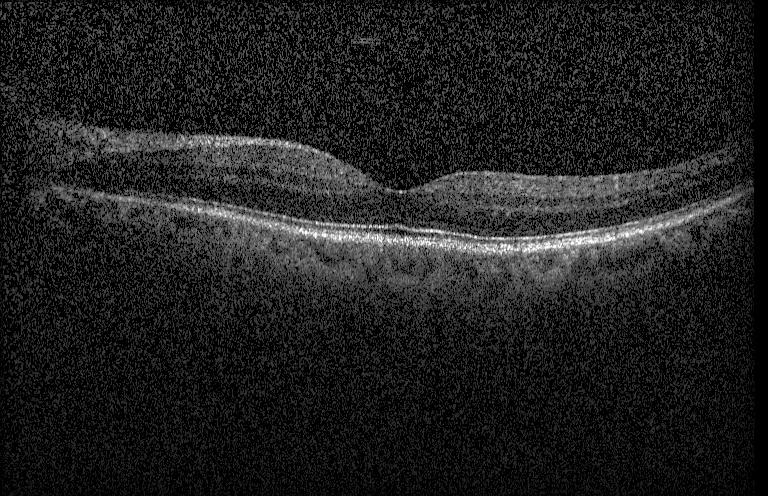

Optical coherence tomography B-scan. OCT finding: no CNV, no DME, and no drusen.